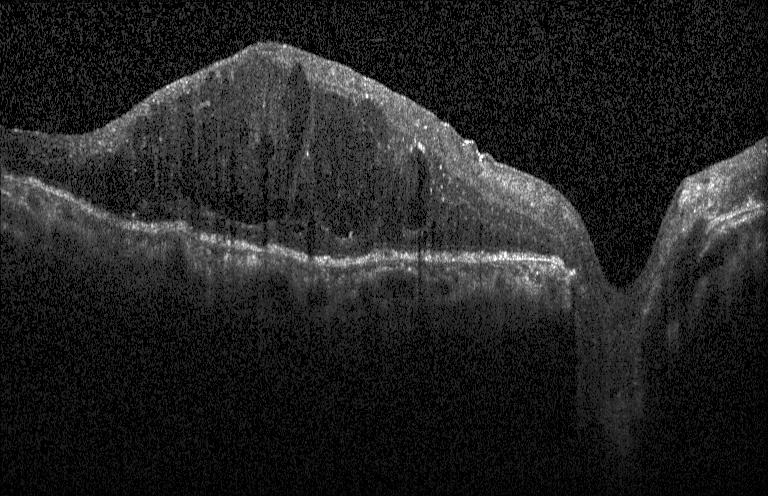

OCT scan showing DME.